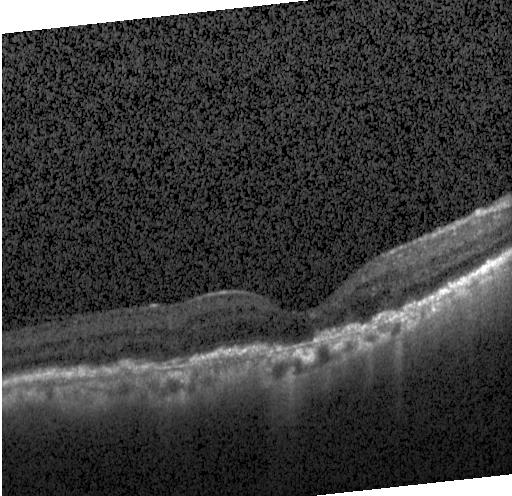 Macular OCT: CNV.